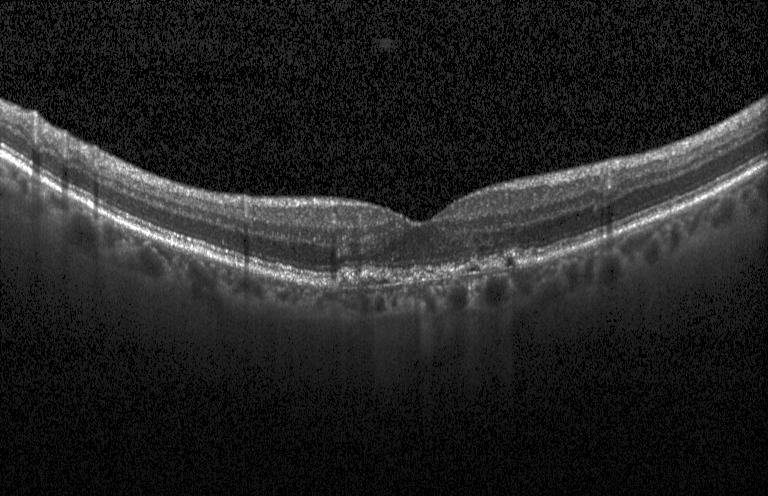 Optical coherence tomography scan — Diagnosis: sub-RPE drusenoid deposits.